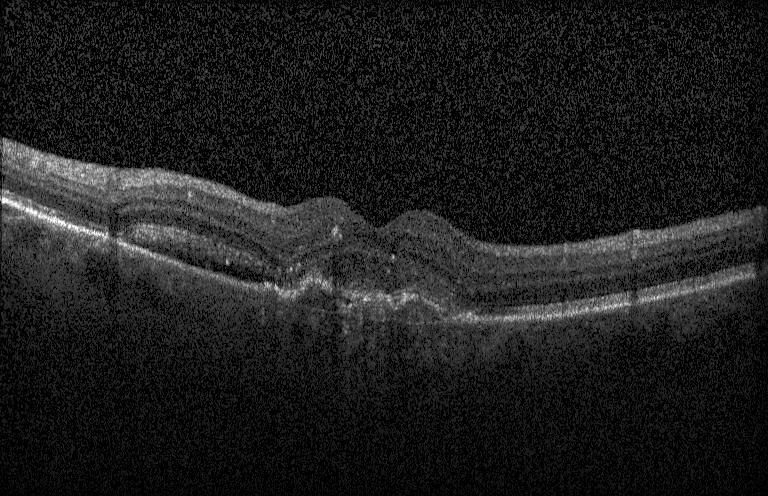
Retinal OCT cross-section.
This B-scan demonstrates a choroidal neovascular membrane.